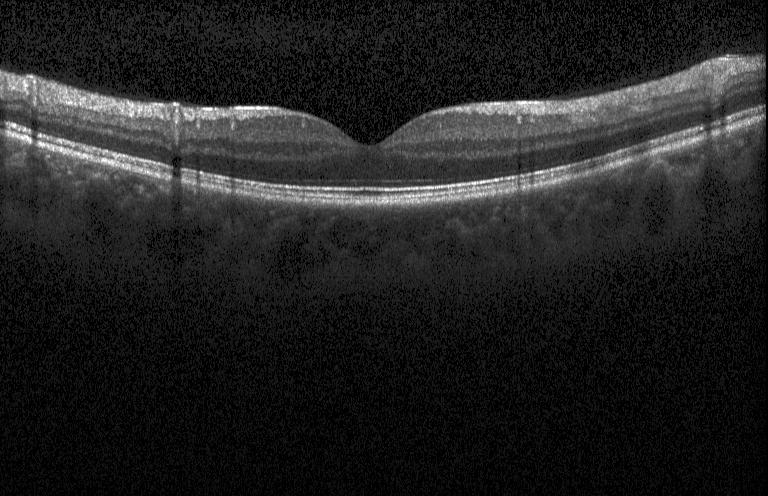
The scan shows no CNV, DME, or drusen.